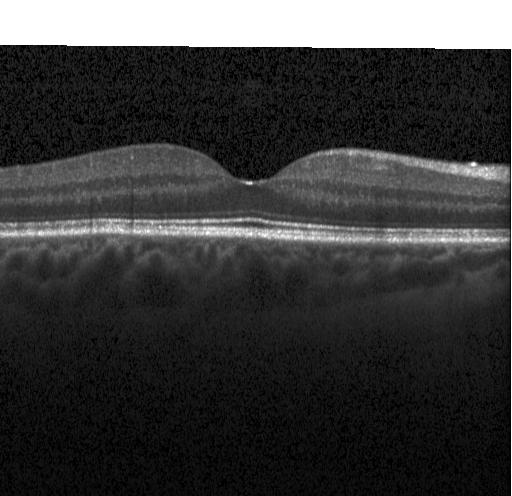

The scan shows no choroidal neovascularization, diabetic macular edema, or drusen.